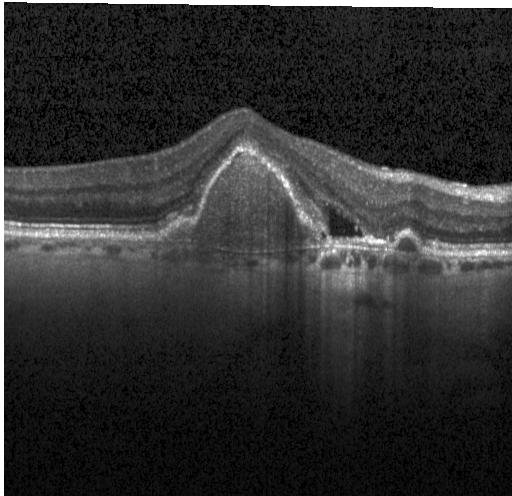 Macular OCT: a choroidal neovascular membrane.